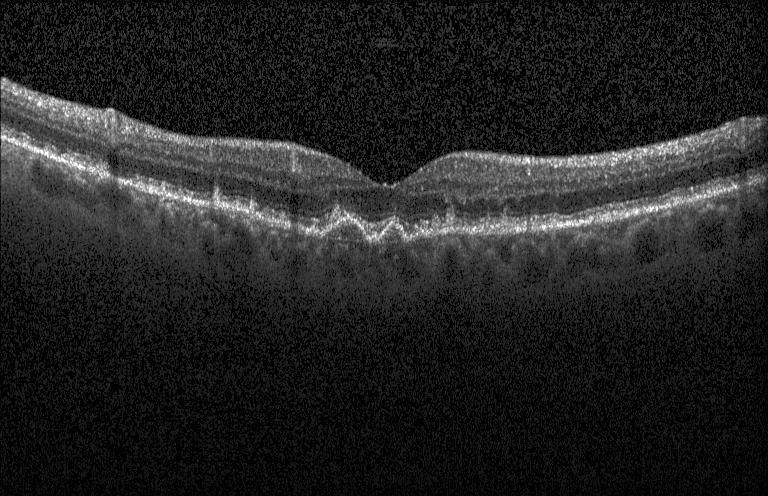 OCT line scan; macular scan; spectral-domain OCT; instrument: Heidelberg Spectralis. Dx: sub-RPE drusenoid deposits.